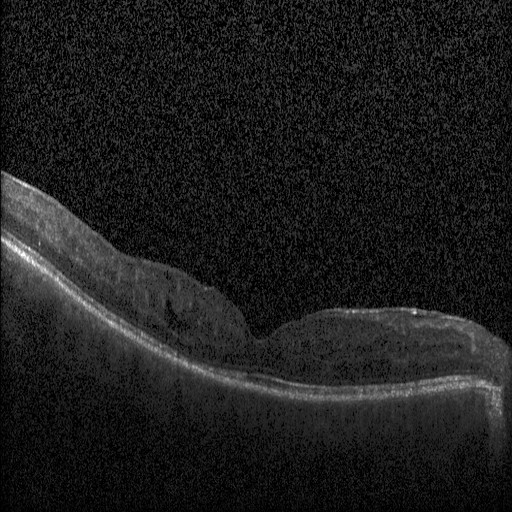 Dx: DME.